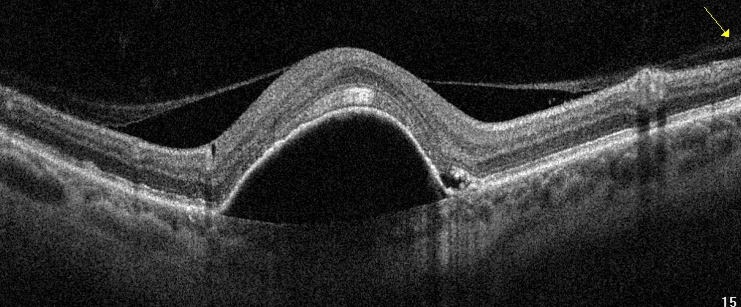 Instrument: Optovue Avanti RTVue XR · retinal OCT B-scan · through the macula — Dx: age-related macular degeneration.